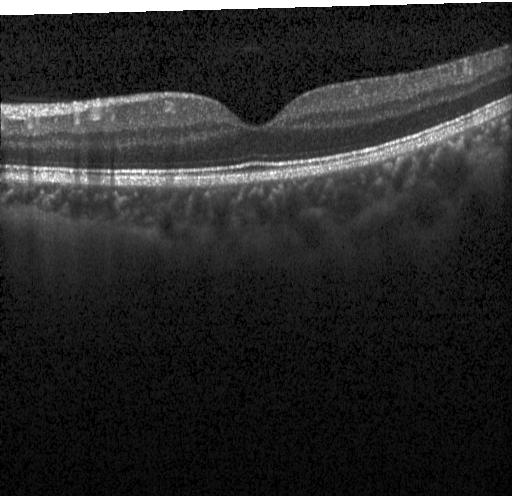
Heidelberg Spectralis. Spectral-domain OCT. Retinal OCT B-scan. Macular scan. Assessment: no evidence of choroidal neovascularization, diabetic macular edema, or drusen.